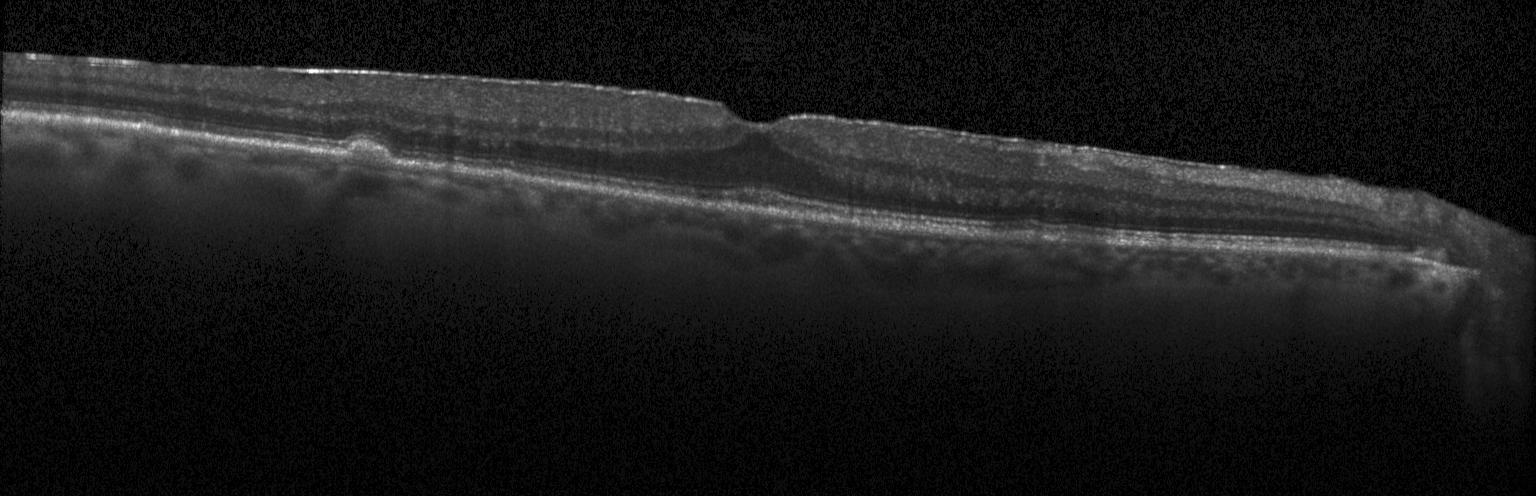 OCT line scan
The scan shows multiple drusen.